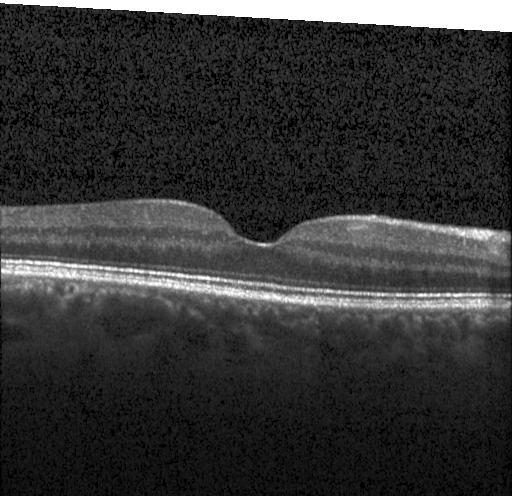
The scan shows neither CNV, DME, nor drusen.